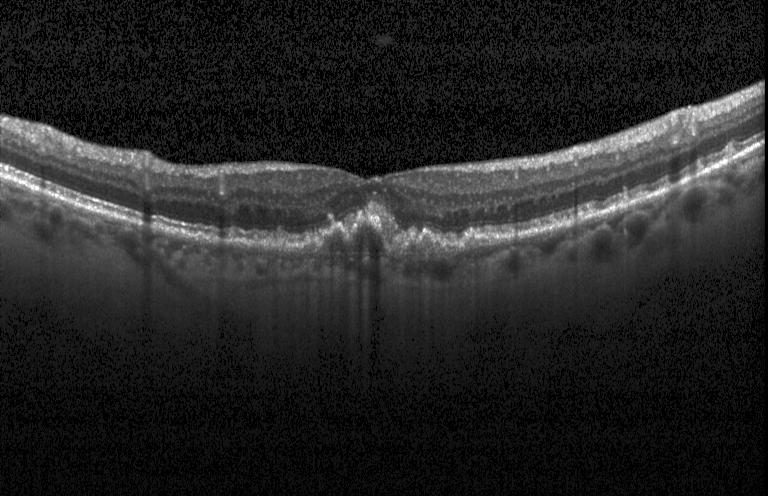 Macular OCT demonstrating choroidal neovascularization (CNV).